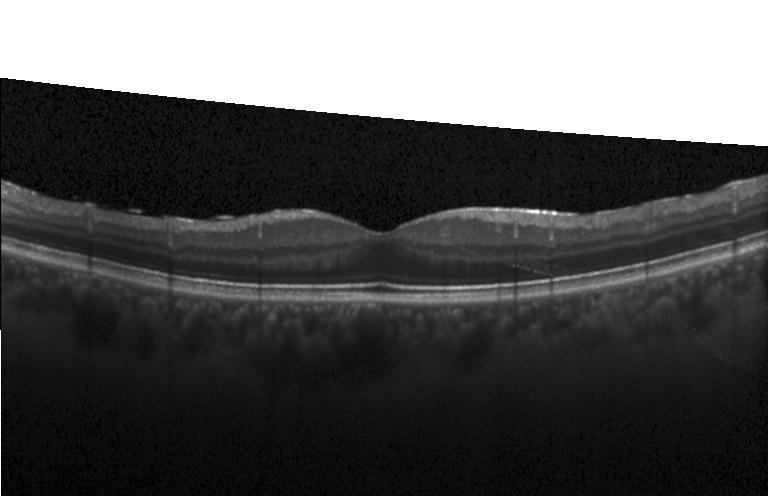

Dx: neither choroidal neovascularization, diabetic macular edema, nor drusen.